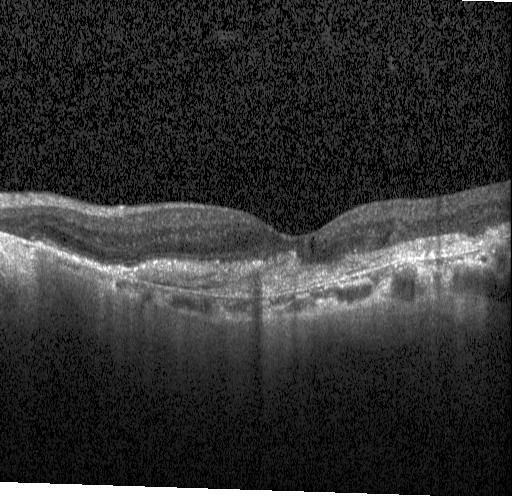

Retinal OCT cross-section, spectral-domain optical coherence tomography, instrument: Heidelberg Spectralis, macular scan. Diagnosis: CNV.